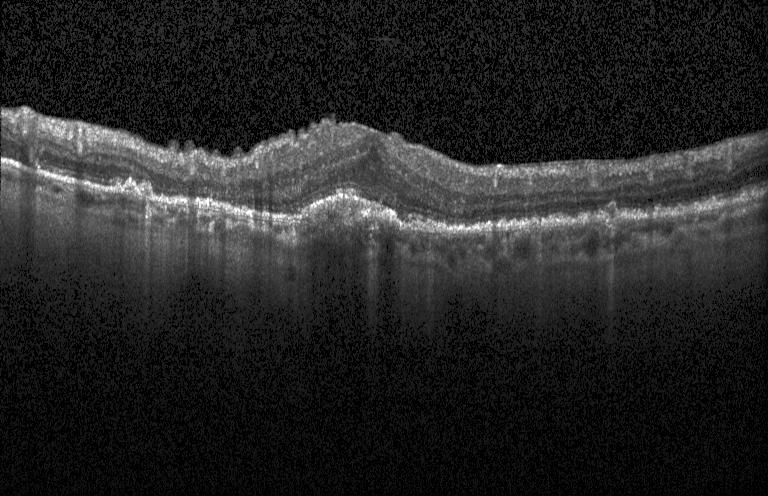

Centered on the fovea; spectral-domain optical coherence tomography; retinal OCT B-scan; Heidelberg Spectralis OCT system — The scan shows choroidal neovascularization.